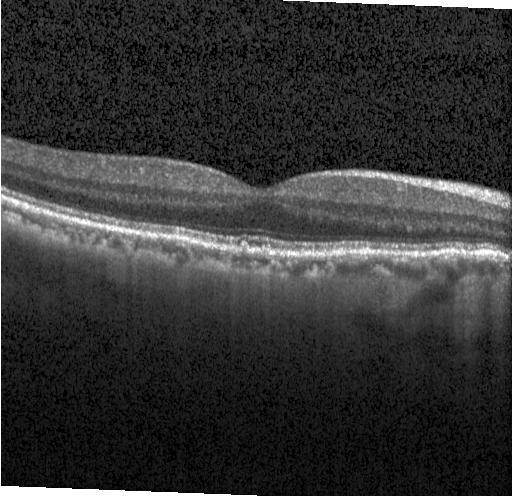

Multiple drusen.